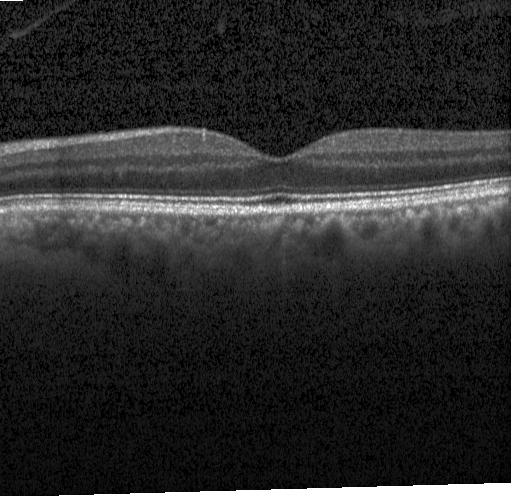

Acquired on a Heidelberg Spectralis · retinal OCT B-scan · through the macula · SD-OCT. Impression: no CNV, no DME, and no drusen.